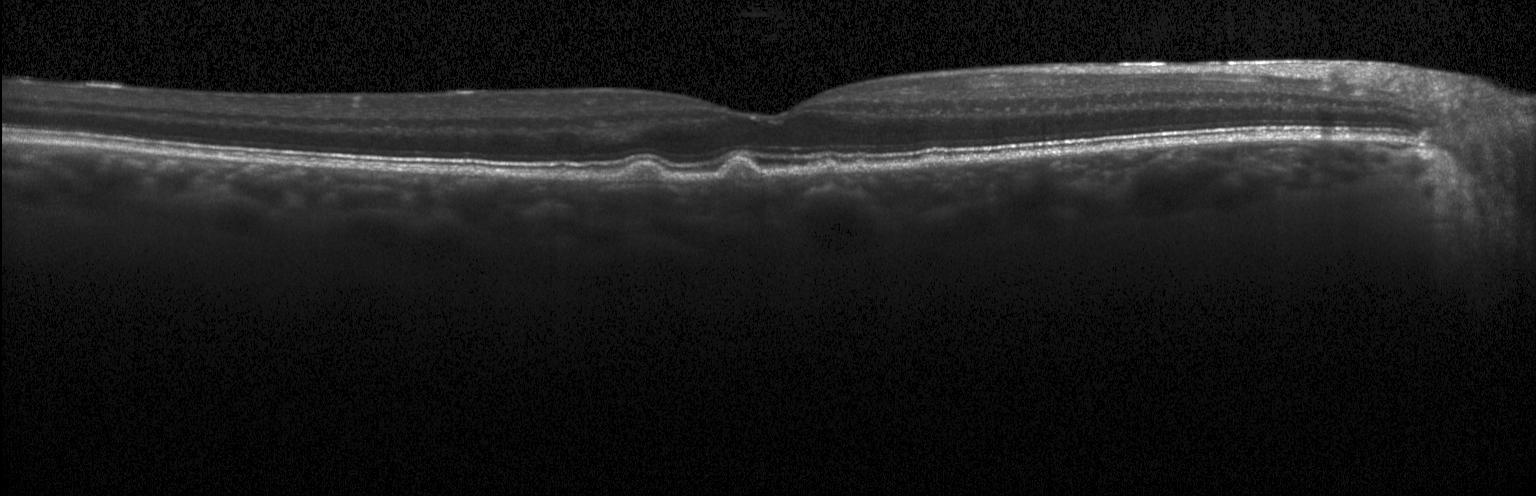

Finding: sub-RPE drusenoid deposits.